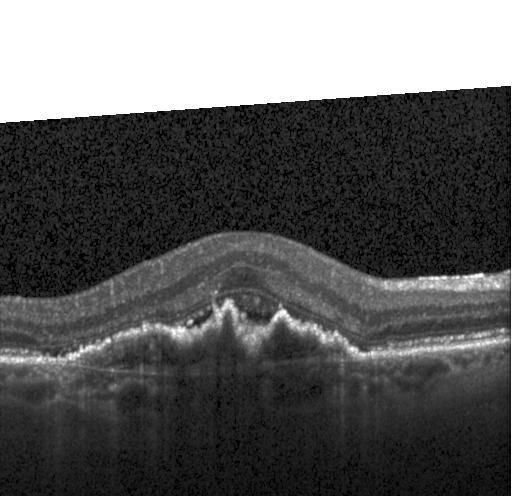
Optical coherence tomography B-scan, acquired on a Heidelberg Spectralis, fovea-centered, SD-OCT.
Finding: choroidal neovascularization (CNV).